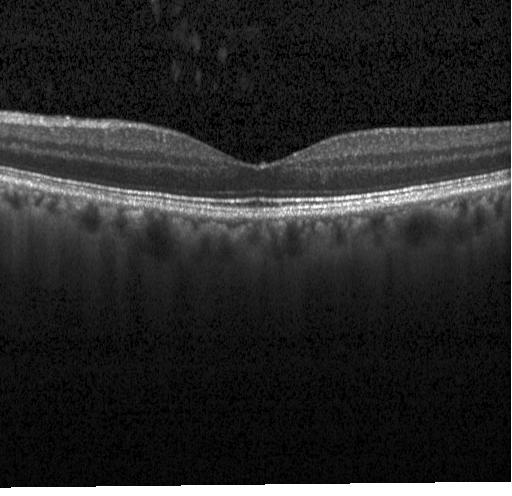
OCT finding: no evidence of CNV, DME, or drusen.